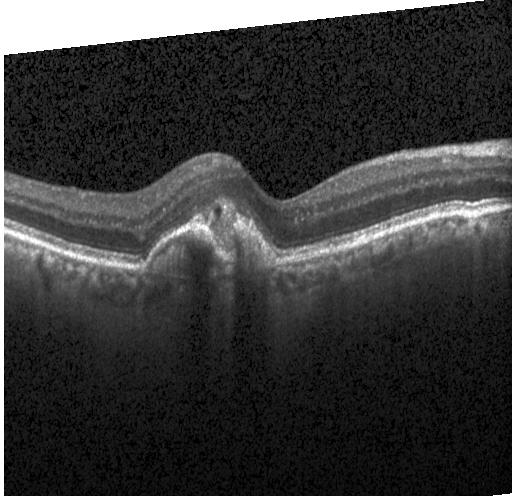
Heidelberg Spectralis. Optical coherence tomography B-scan.
Impression: a choroidal neovascular membrane.